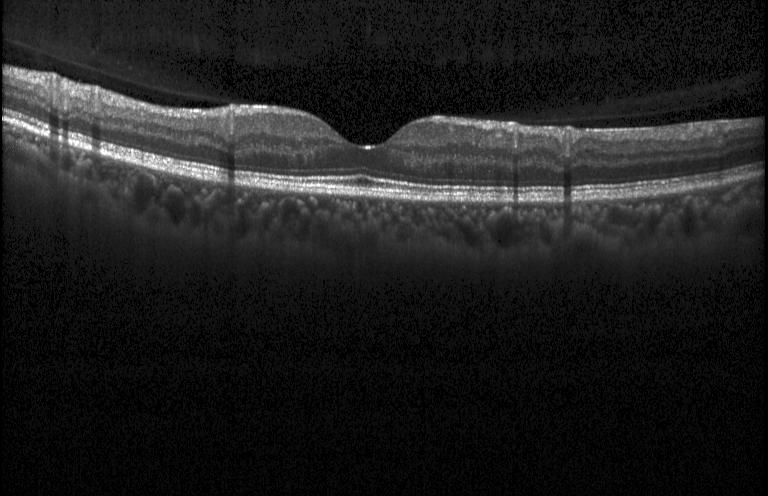
Retinal OCT cross-section showing neither CNV, DME, nor drusen.